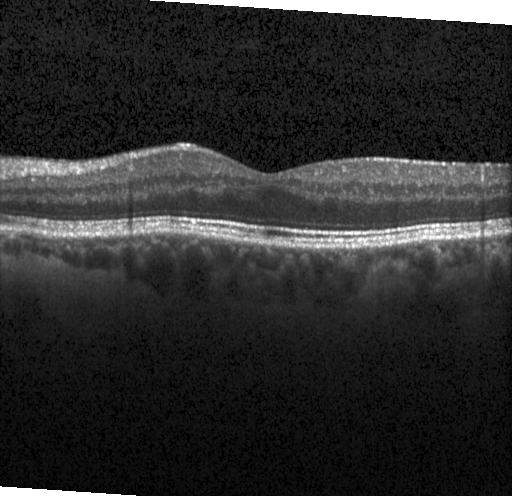
Finding: no choroidal neovascularization, no diabetic macular edema, and no drusen.